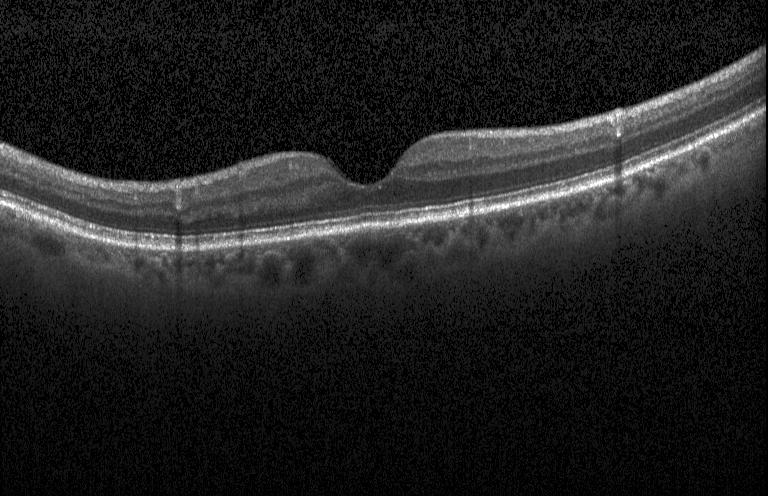 Retinal OCT cross-section showing no choroidal neovascularization, diabetic macular edema, or drusen.